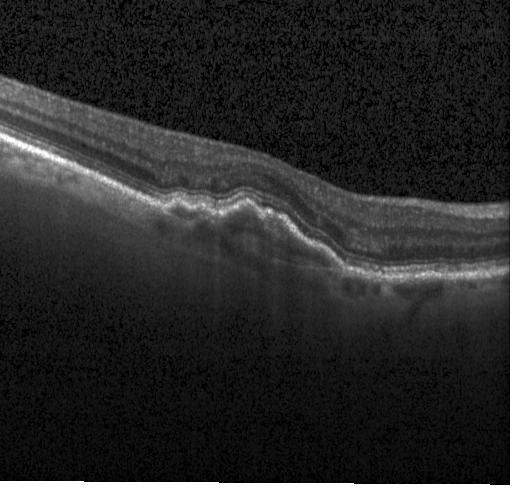 Finding: choroidal neovascularization.